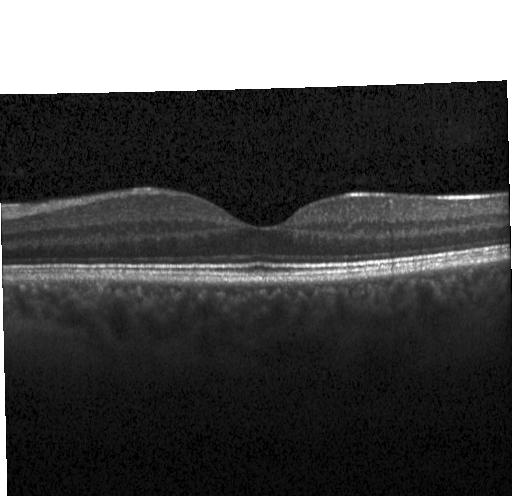 Optical coherence tomography B-scan; SD-OCT
Neither CNV, DME, nor drusen.